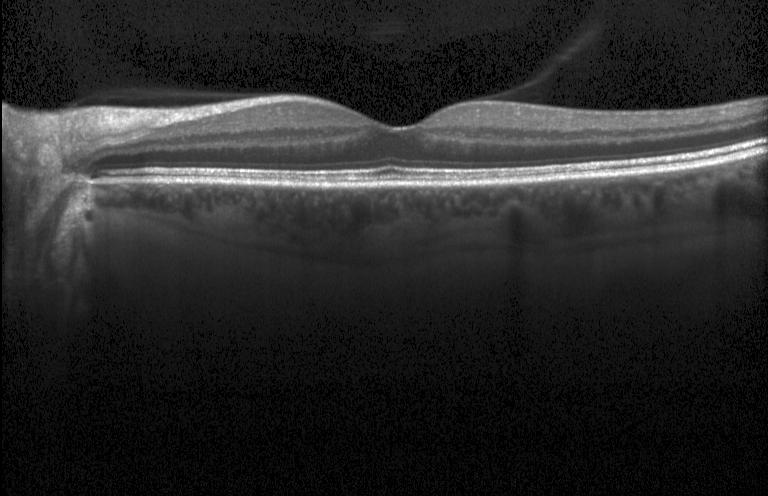 Diagnosis: no choroidal neovascularization, no diabetic macular edema, and no drusen.